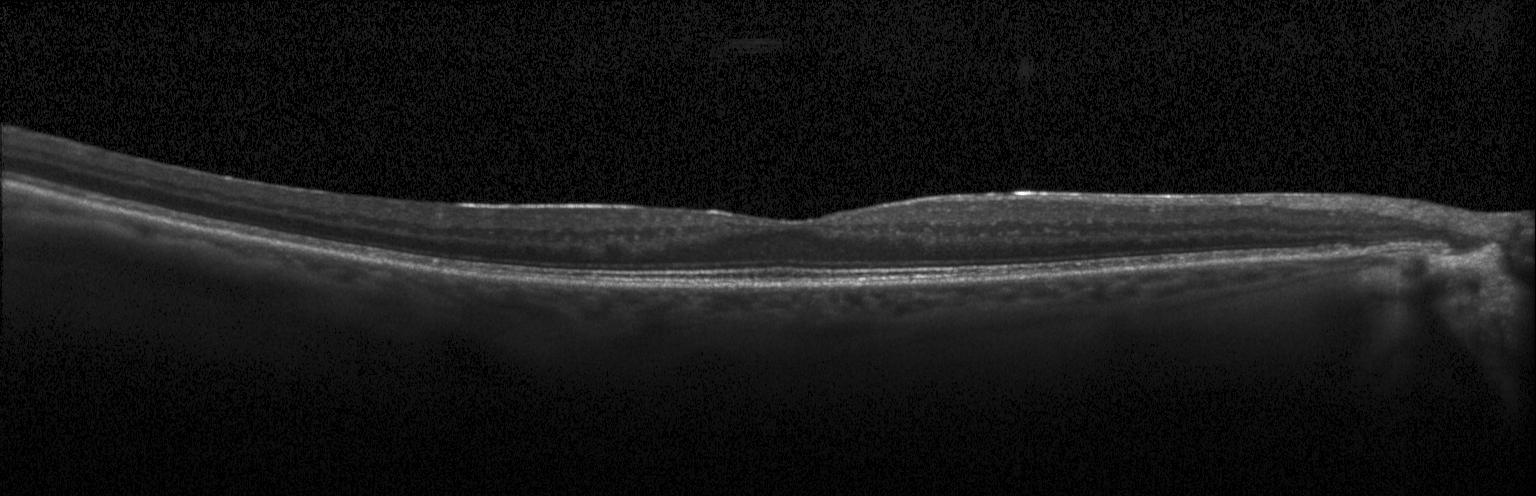

Retinal OCT cross-section. Diagnosis: no evidence of choroidal neovascularization, diabetic macular edema, or drusen.